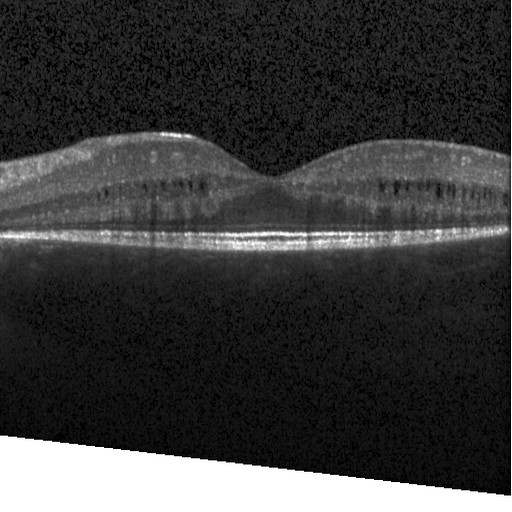
Spectral-domain OCT B-scan: DME.